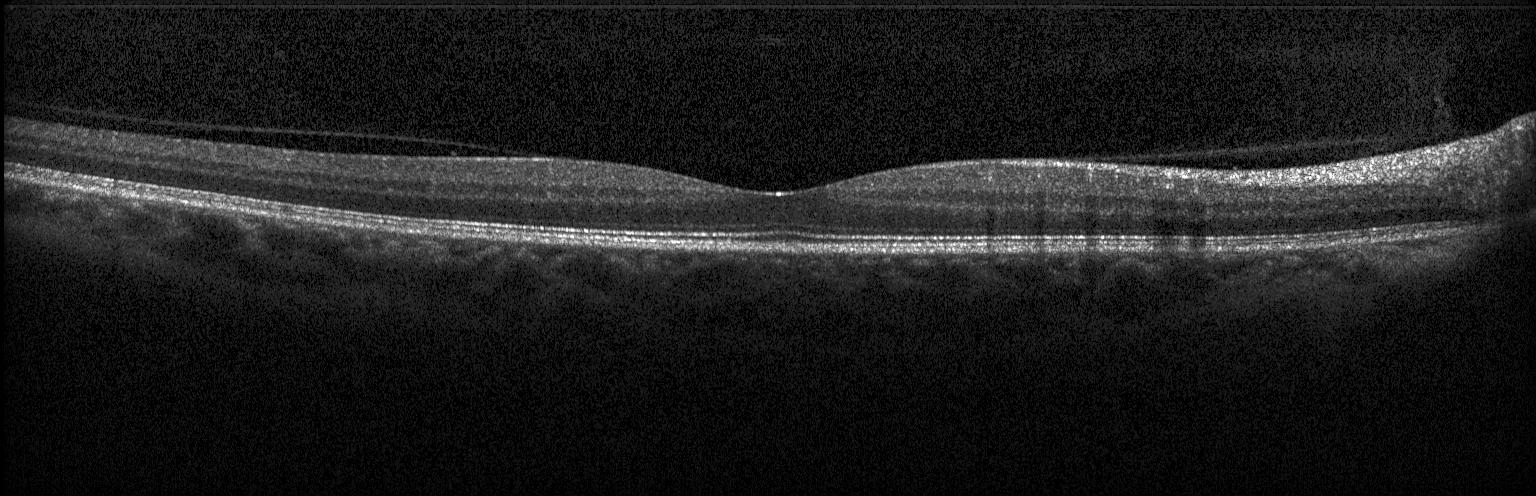 Heidelberg Spectralis, retinal OCT B-scan, horizontal scan through the fovea.
Diagnosis: no CNV, DME, or drusen.